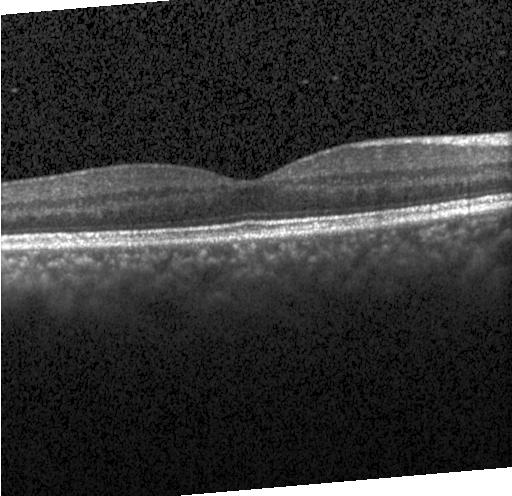

Fovea-centered; OCT line scan — This B-scan demonstrates no choroidal neovascularization, no diabetic macular edema, and no drusen.